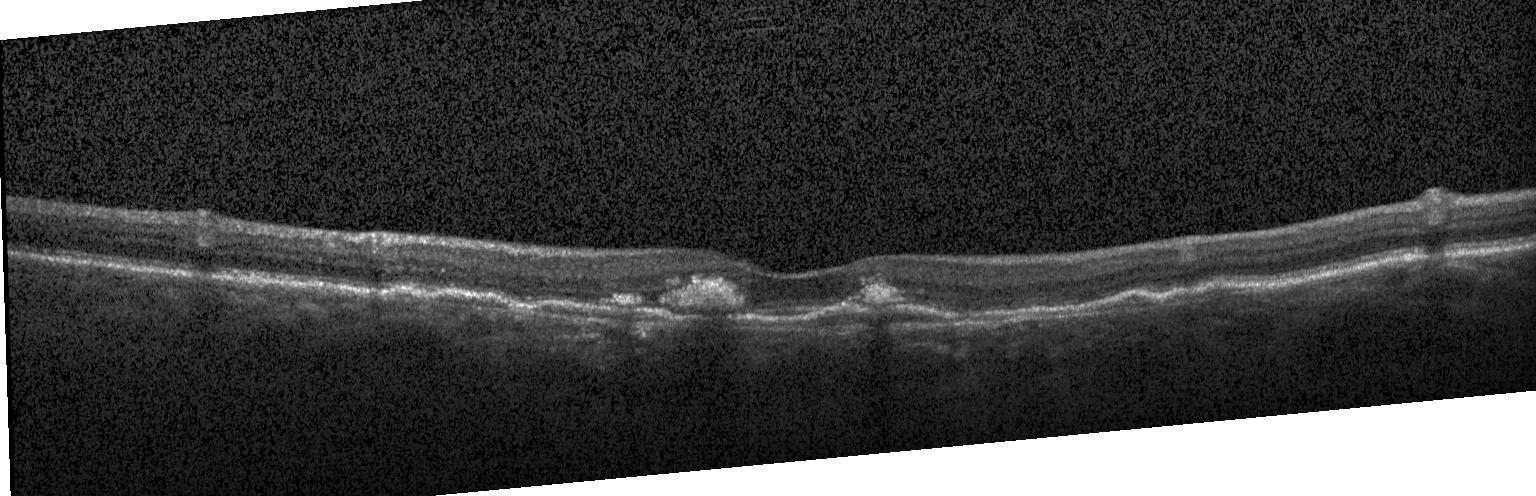

Spectral-domain OCT B-scan: a choroidal neovascular membrane.